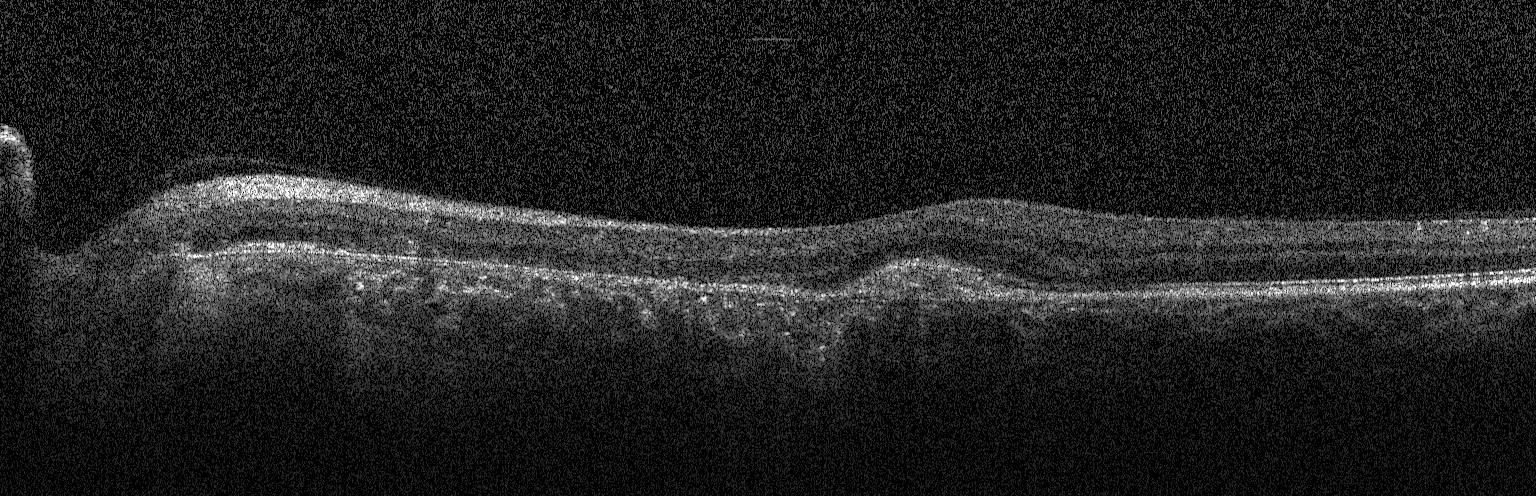

Macular OCT demonstrating CNV.